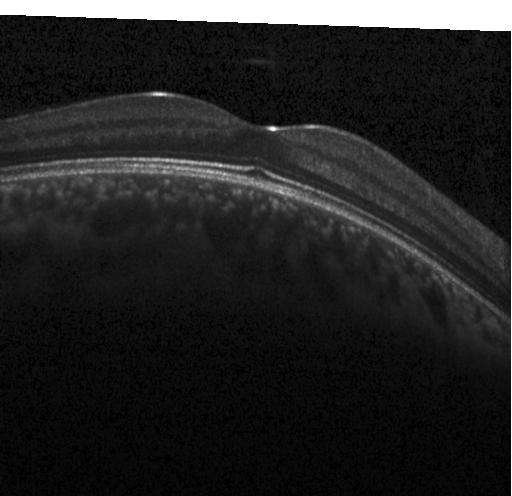 SD-OCT, optical coherence tomography B-scan. Impression: no CNV, no DME, and no drusen.